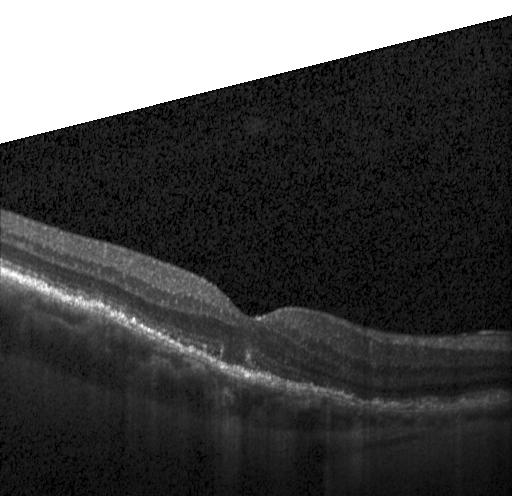
Spectral-domain OCT B-scan: a choroidal neovascular membrane.